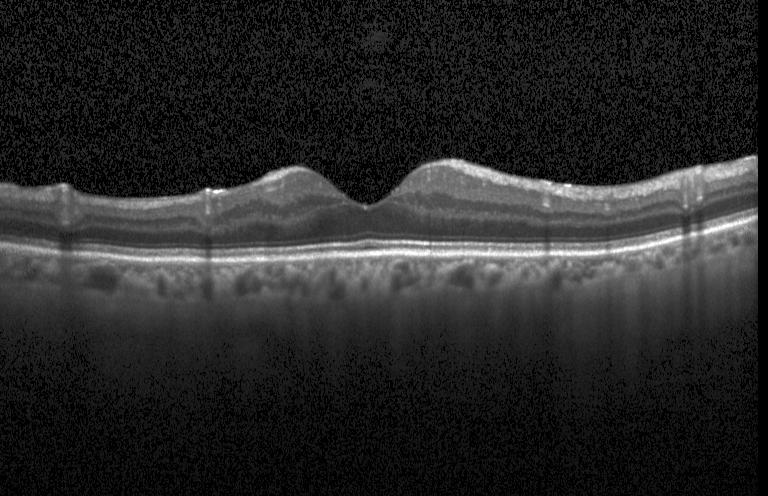 Spectral-domain optical coherence tomography. OCT line scan. Centered on the fovea.
Finding: no choroidal neovascularization, diabetic macular edema, or drusen.